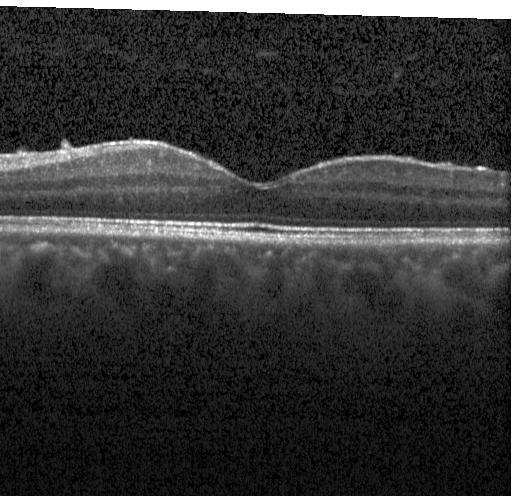 OCT line scan
The scan shows no evidence of choroidal neovascularization, diabetic macular edema, or drusen.